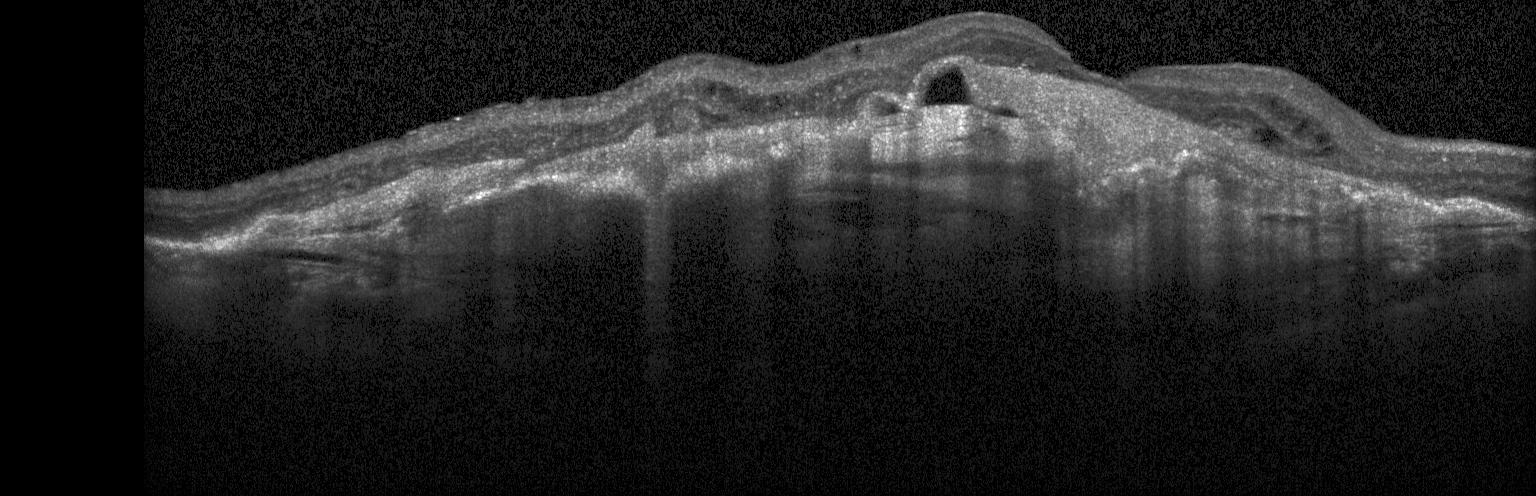
OCT B-scan.
Impression: choroidal neovascularization (CNV).